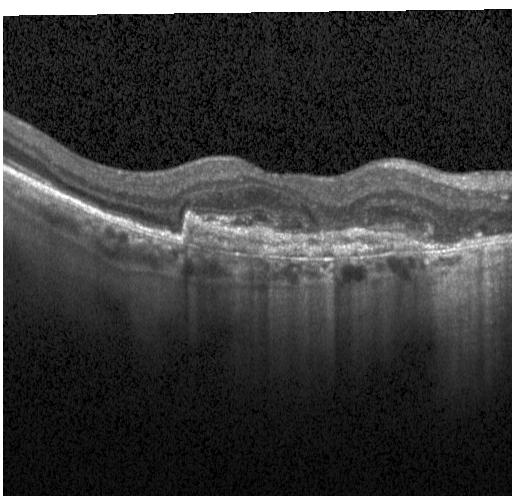
Dx: CNV.